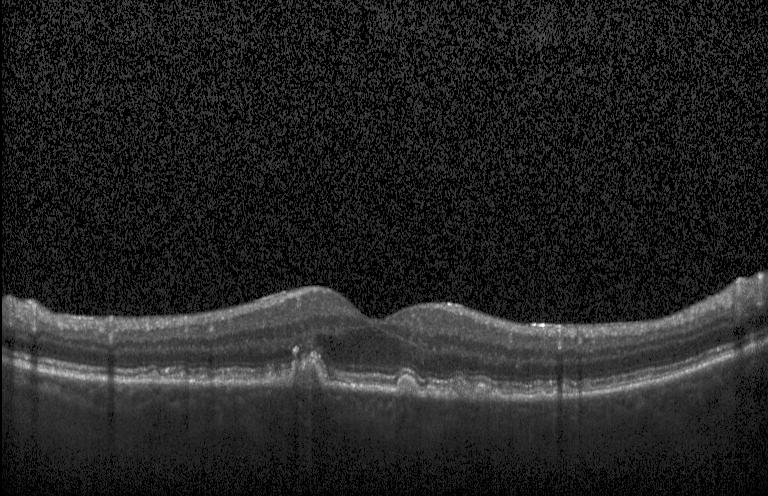
Impression: multiple drusen.